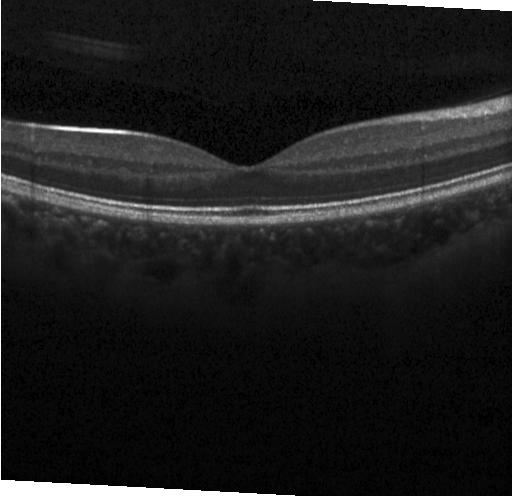

Instrument: Heidelberg Spectralis · SD-OCT · optical coherence tomography scan · horizontal scan through the fovea. The scan shows neither choroidal neovascularization, diabetic macular edema, nor drusen.